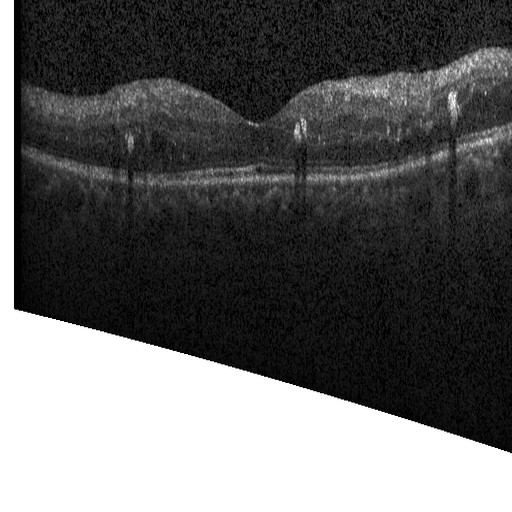 Retinal OCT B-scan · Heidelberg Spectralis — Macular OCT: diabetic macular edema (DME).